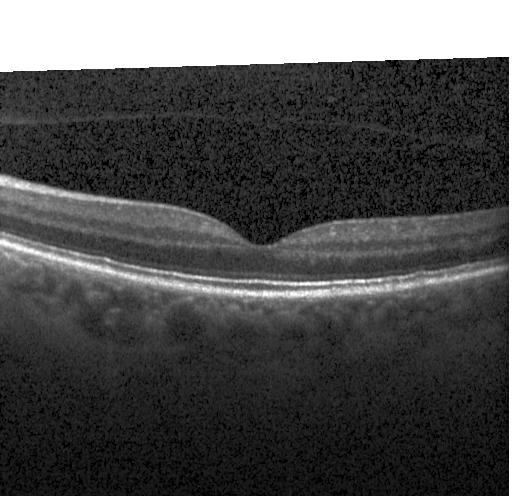 Macular OCT demonstrating no choroidal neovascularization, no diabetic macular edema, and no drusen.